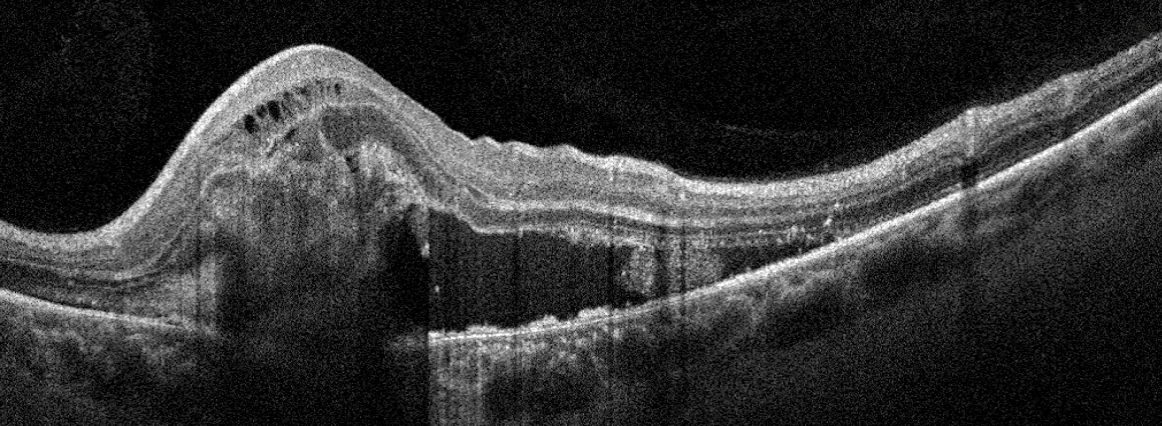
OCT B-scan · oculus sinister
Finding: age-related macular degeneration (AMD).